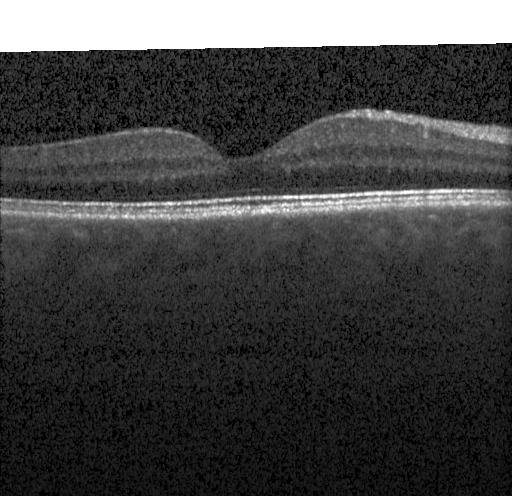 OCT finding: no choroidal neovascularization, no diabetic macular edema, and no drusen.